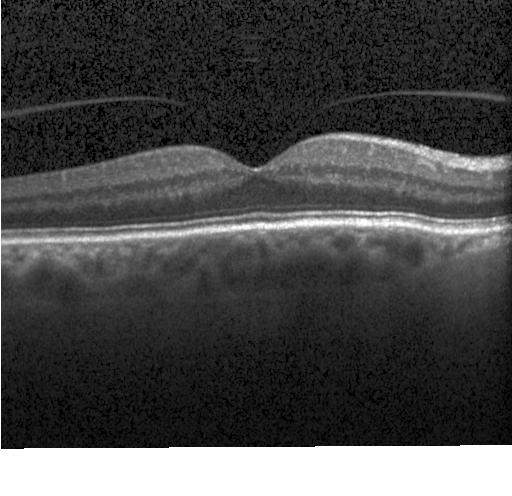
Retinal OCT cross-section showing neither choroidal neovascularization, diabetic macular edema, nor drusen.